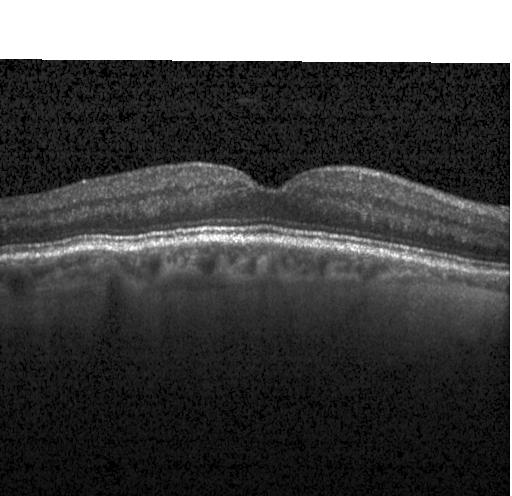 Heidelberg Spectralis OCT system · OCT B-scan · through the macula · spectral-domain OCT — Macular OCT: no choroidal neovascularization, no diabetic macular edema, and no drusen.